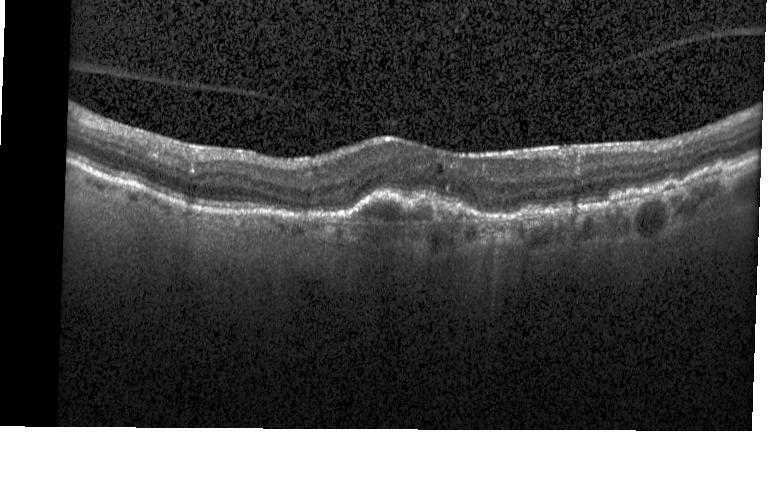

Choroidal neovascularization (CNV).